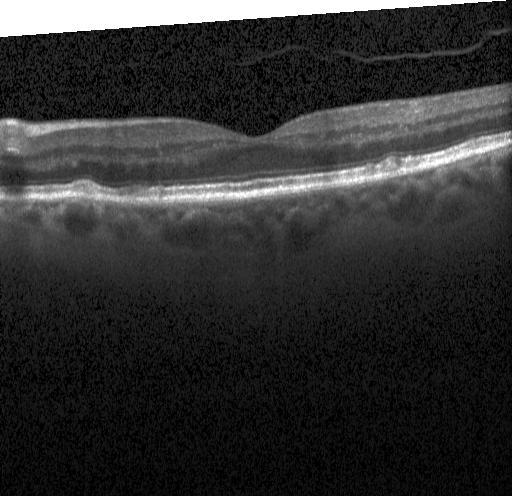

Macular OCT: drusen.